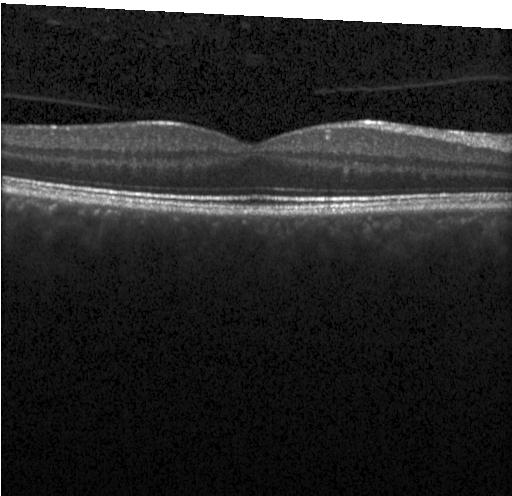

Impression: neither choroidal neovascularization, diabetic macular edema, nor drusen.